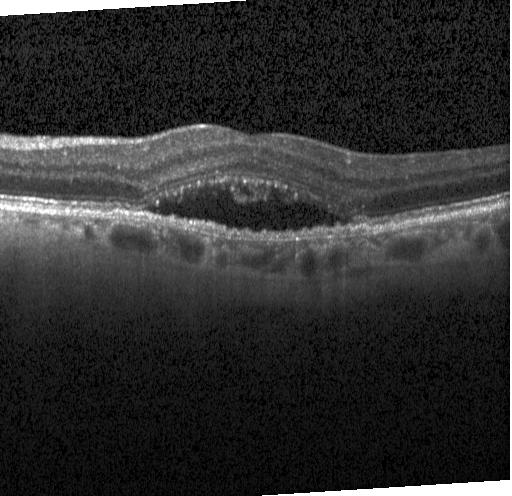

OCT line scan.
Finding: a choroidal neovascular membrane.